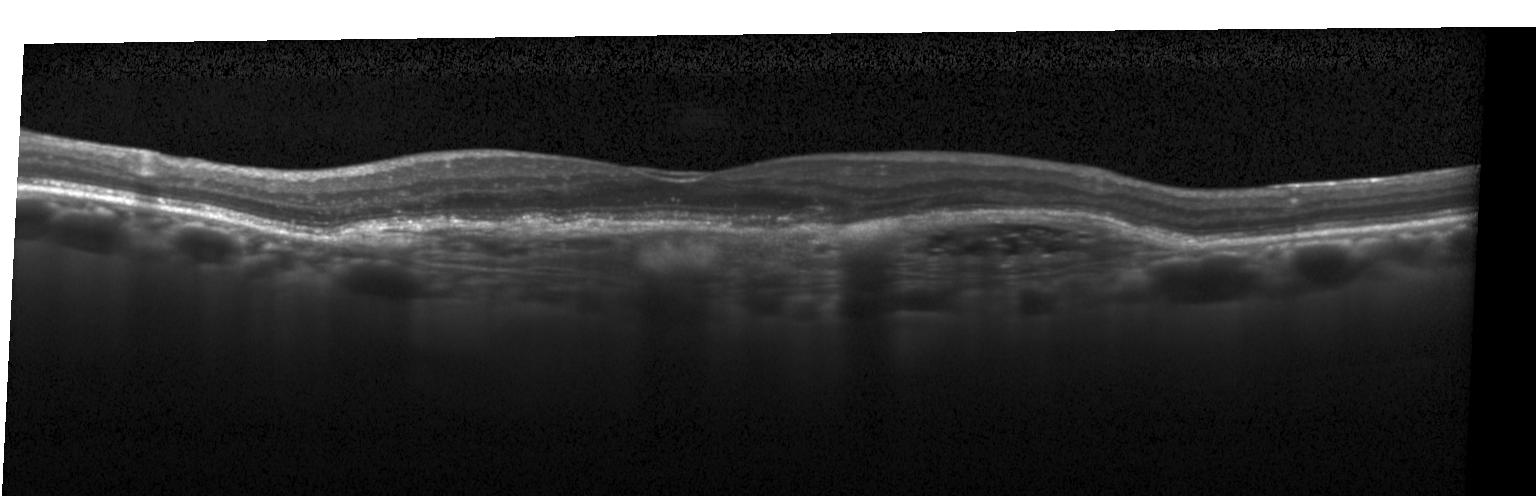 Finding: choroidal neovascularization.